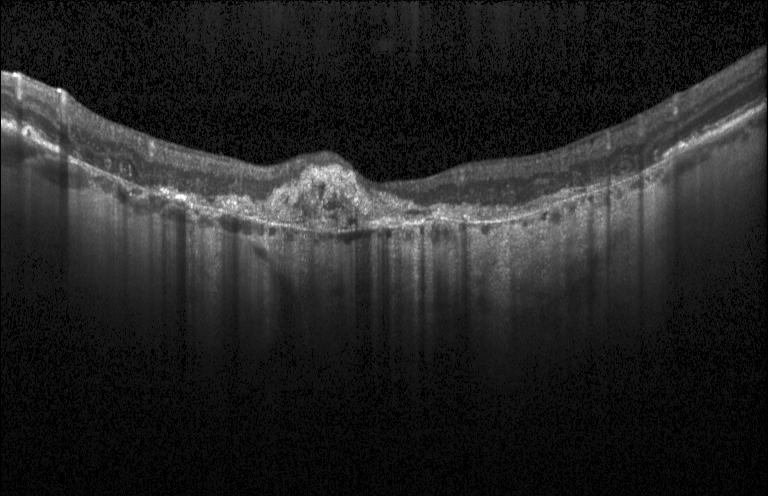
OCT line scan
OCT finding: a choroidal neovascular membrane.